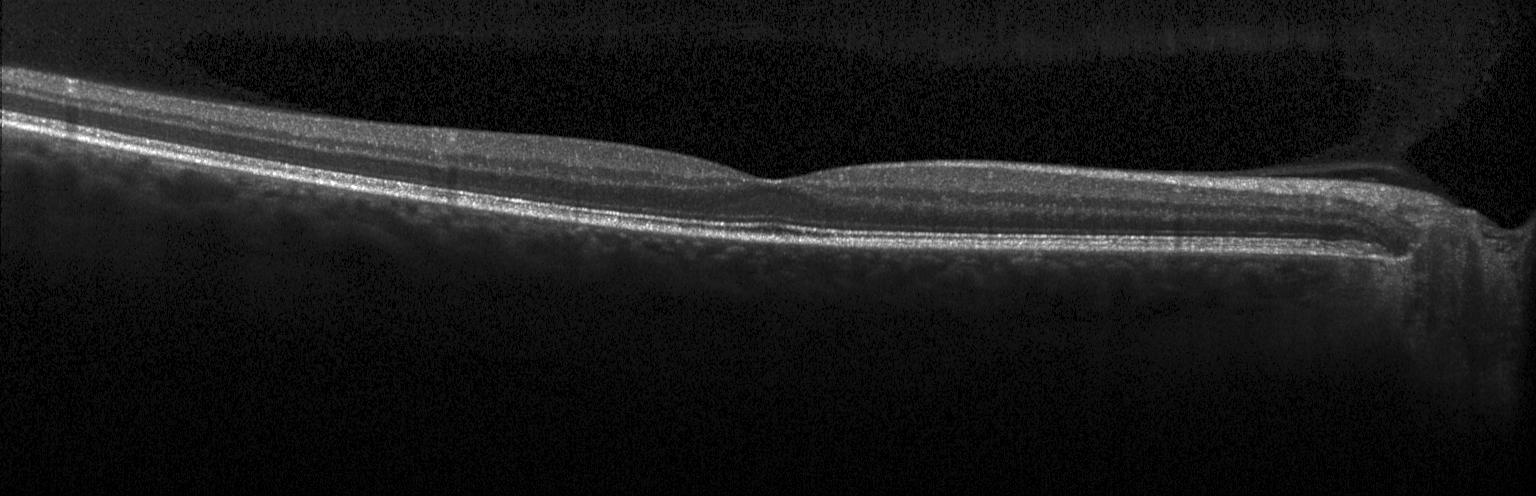 Spectral-domain OCT; optical coherence tomography B-scan; instrument: Heidelberg Spectralis; horizontal scan through the fovea — Assessment: no choroidal neovascularization, no diabetic macular edema, and no drusen.